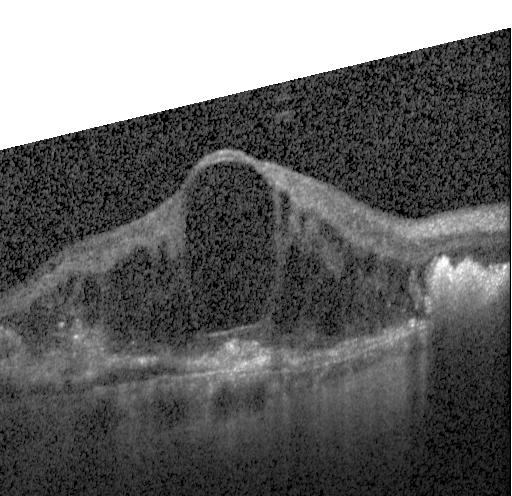 Heidelberg Spectralis OCT system · centered on the fovea · retinal OCT B-scan.
Assessment: a choroidal neovascular membrane.